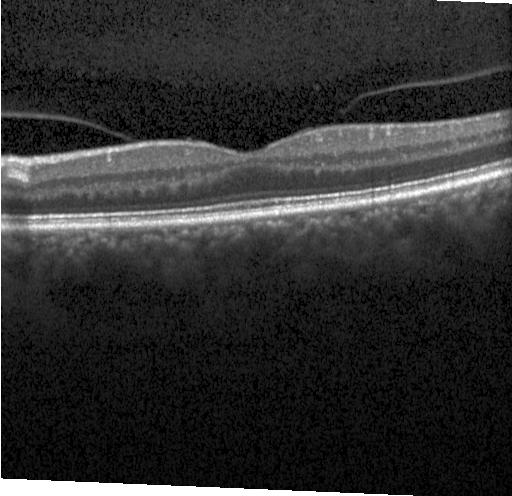

This B-scan demonstrates no CNV, no DME, and no drusen.